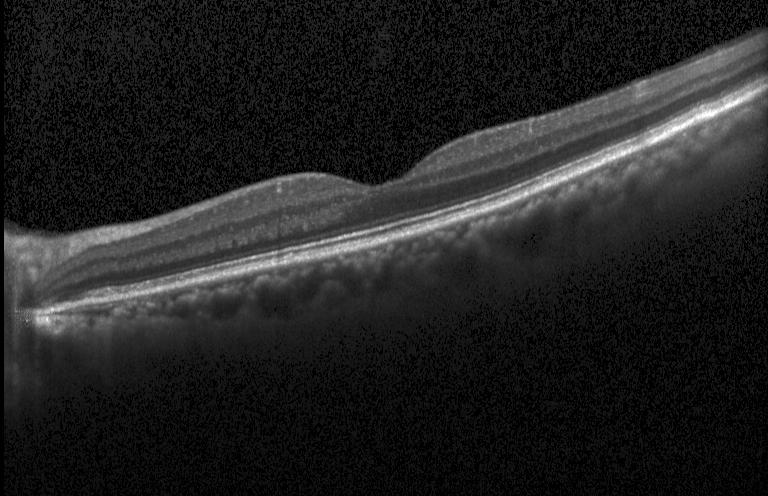

Spectral-domain OCT. Acquired on a Heidelberg Spectralis. Optical coherence tomography B-scan
Impression: neither choroidal neovascularization, diabetic macular edema, nor drusen.